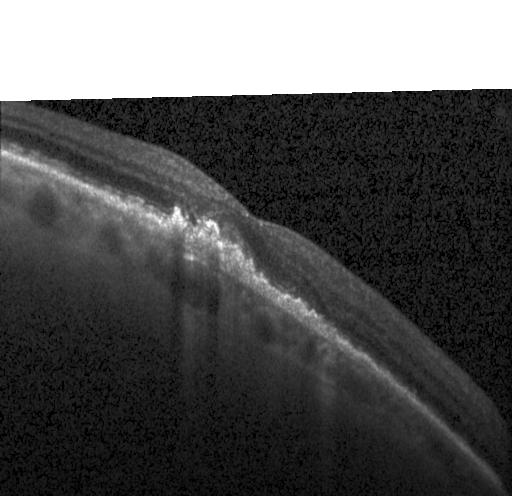 Impression: choroidal neovascularization (CNV).